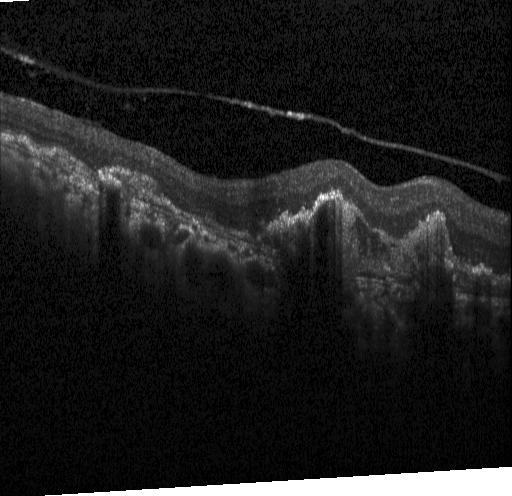

Choroidal neovascularization.